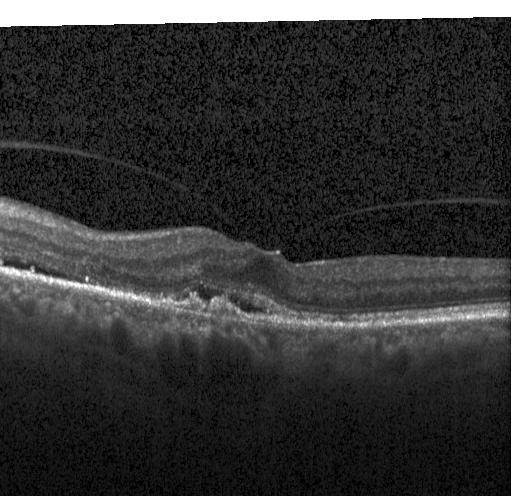
Instrument: Heidelberg Spectralis · optical coherence tomography B-scan — Finding: CNV.